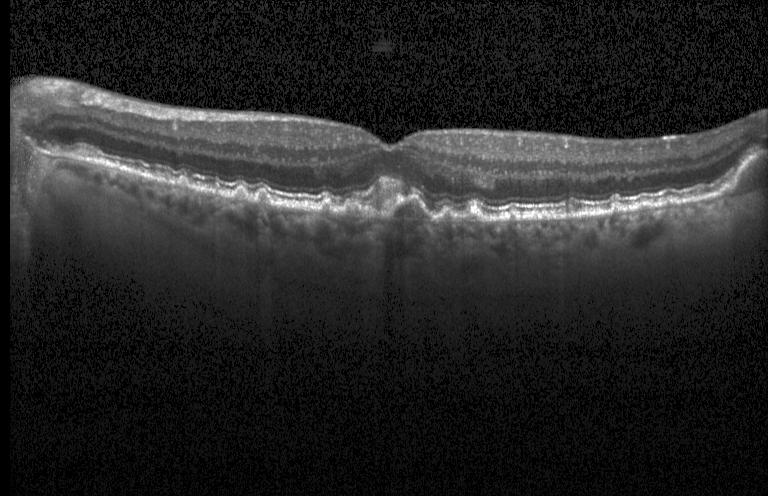

This B-scan demonstrates a choroidal neovascular membrane.